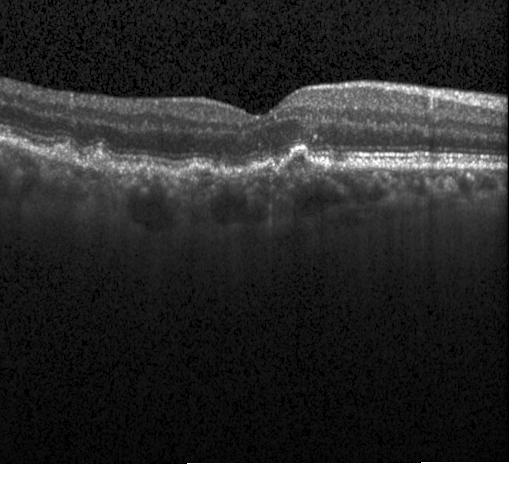

OCT line scan. Finding: multiple drusen.